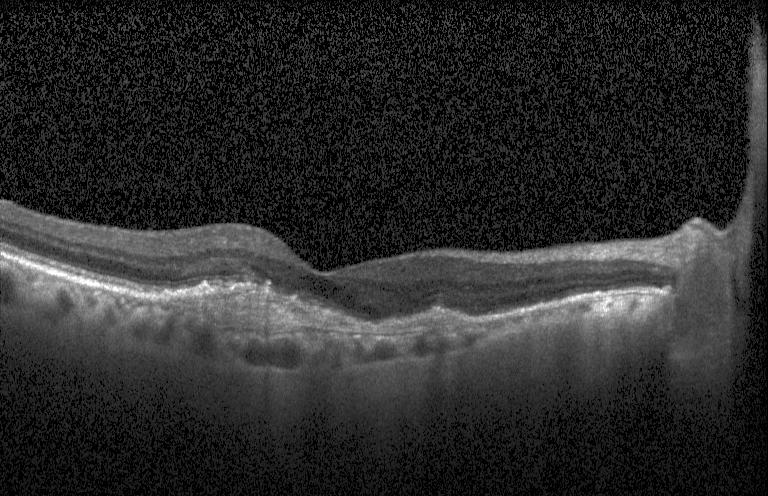
Retinal OCT cross-section showing a choroidal neovascular membrane.